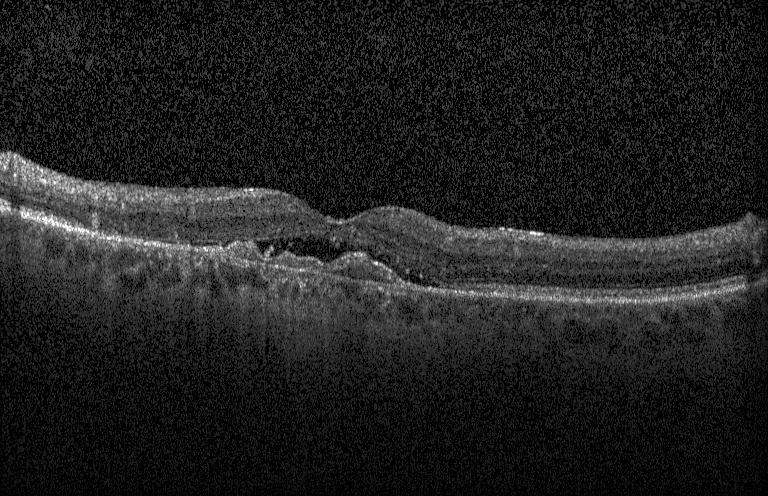

Optical coherence tomography scan
This B-scan demonstrates choroidal neovascularization.